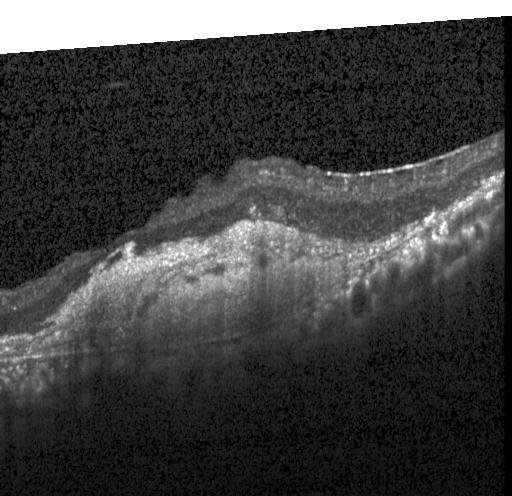
Spectral-domain optical coherence tomography · optical coherence tomography scan · centered on the fovea · acquired on a Heidelberg Spectralis
Impression: a choroidal neovascular membrane.